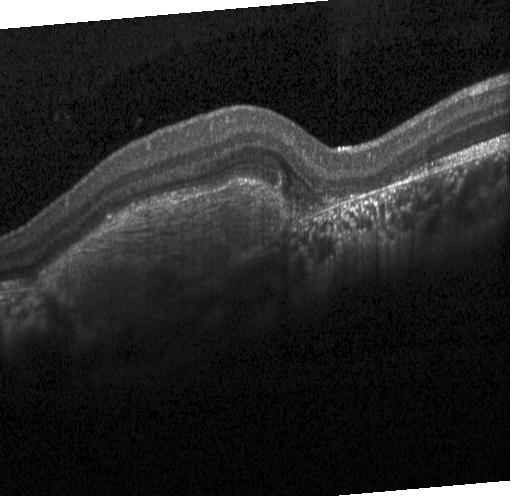
Centered on the fovea. Optical coherence tomography B-scan. Spectral-domain OCT
Dx: choroidal neovascularization.